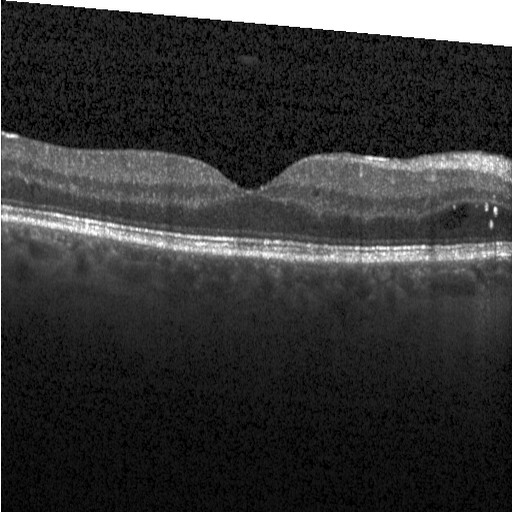

OCT B-scan; Heidelberg Spectralis — Assessment: diabetic macular edema (DME).